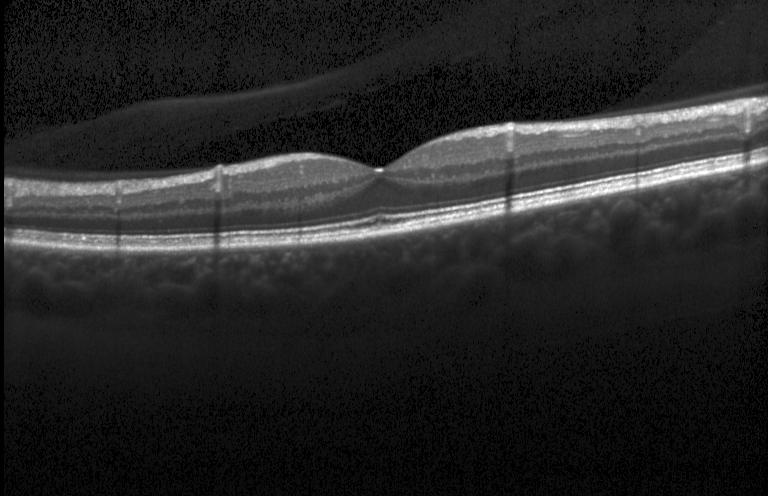

Heidelberg Spectralis OCT system. SD-OCT. Fovea-centered. OCT B-scan — This B-scan demonstrates neither CNV, DME, nor drusen.